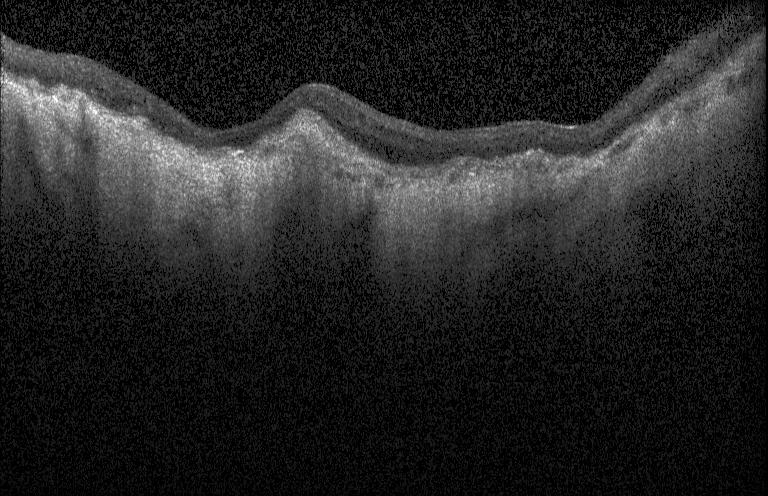 Diagnosis: choroidal neovascularization.